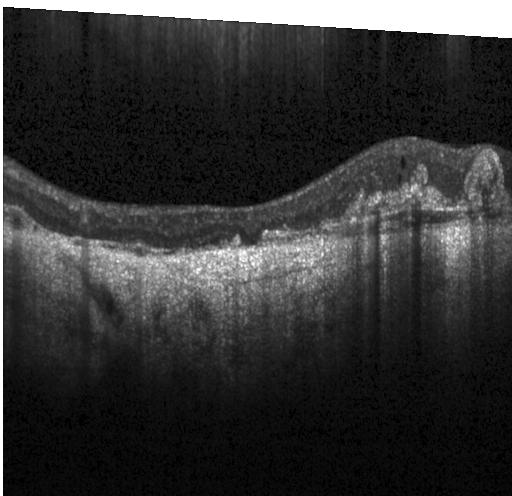

Optical coherence tomography B-scan
Diagnosis: a choroidal neovascular membrane.